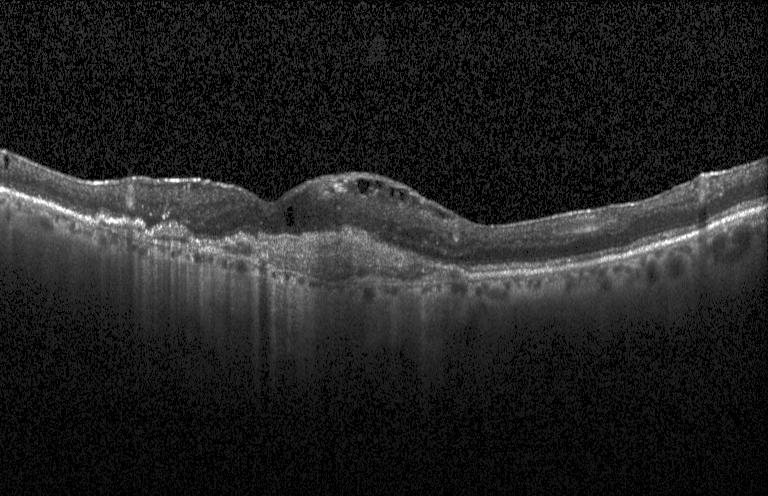 Spectral-domain OCT B-scan: choroidal neovascularization.